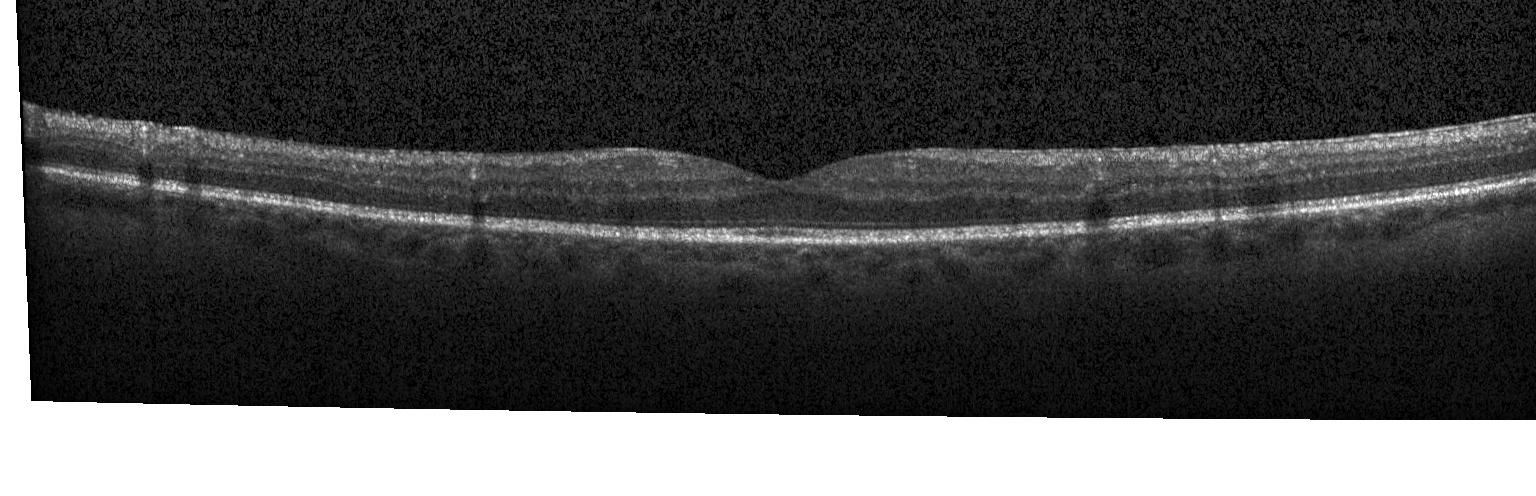

Spectral-domain OCT; retinal OCT B-scan. Assessment: neither choroidal neovascularization, diabetic macular edema, nor drusen.